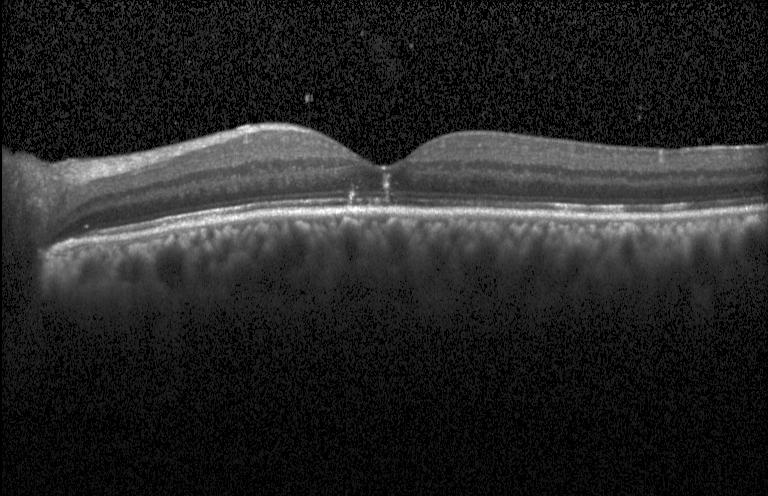
Retinal OCT cross-section; horizontal scan through the fovea; spectral-domain OCT.
Diagnosis: no choroidal neovascularization, diabetic macular edema, or drusen.